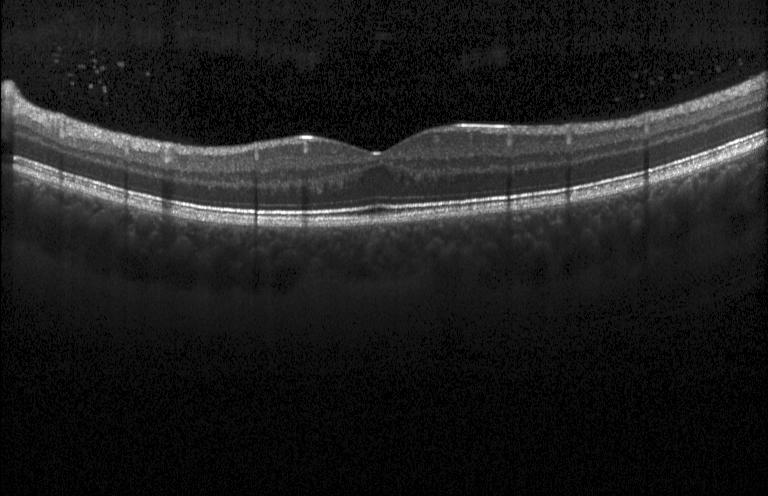
Finding: neither choroidal neovascularization, diabetic macular edema, nor drusen.